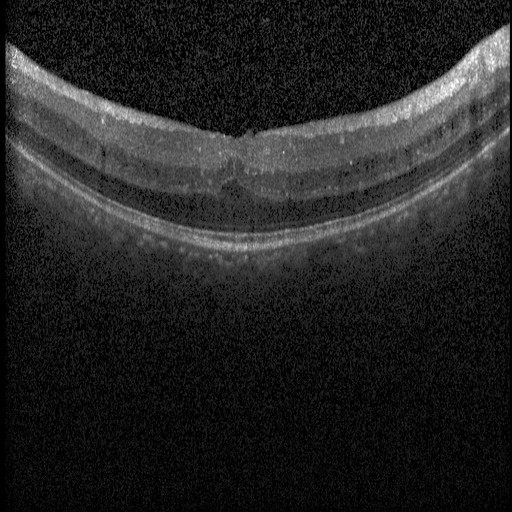 SD-OCT. Retinal OCT B-scan. Instrument: Heidelberg Spectralis. Macular scan.
Finding: DME.